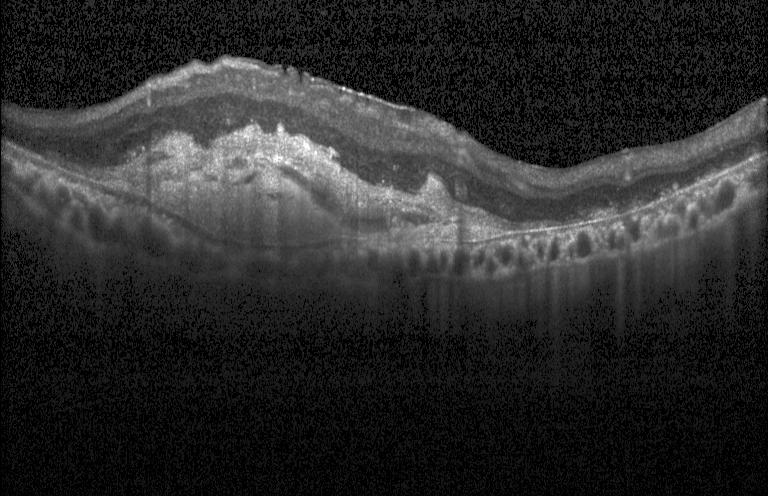

Retinal OCT cross-section · instrument: Heidelberg Spectralis · SD-OCT — OCT finding: choroidal neovascularization.